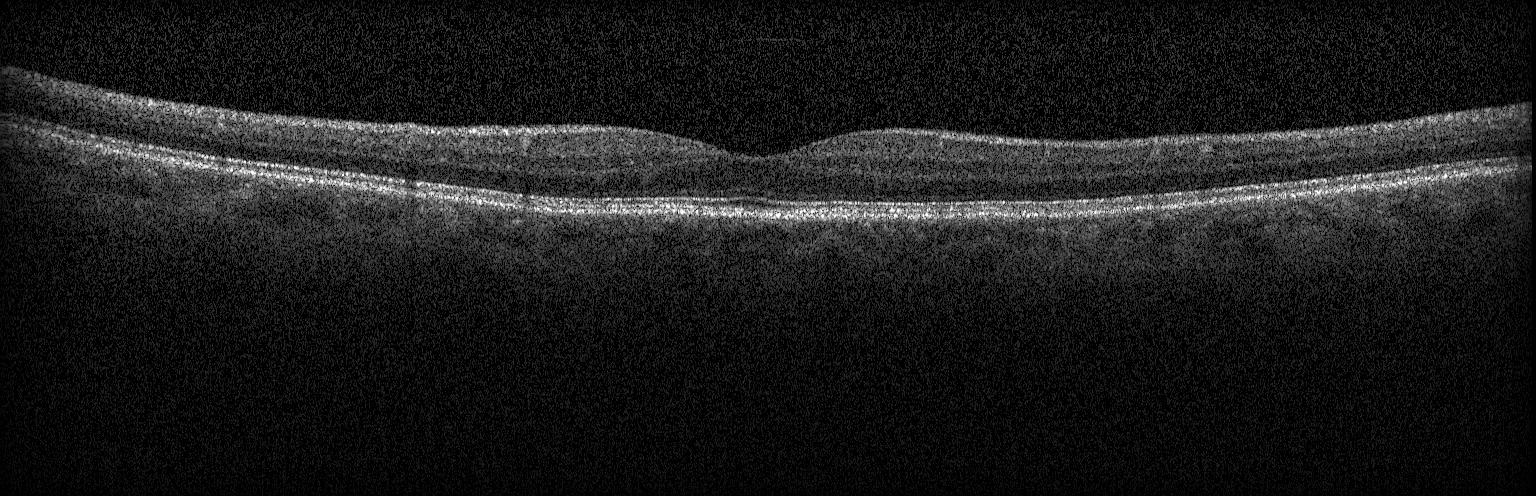
Acquired on a Heidelberg Spectralis · optical coherence tomography scan · spectral-domain OCT · horizontal scan through the fovea — This B-scan demonstrates neither choroidal neovascularization, diabetic macular edema, nor drusen.